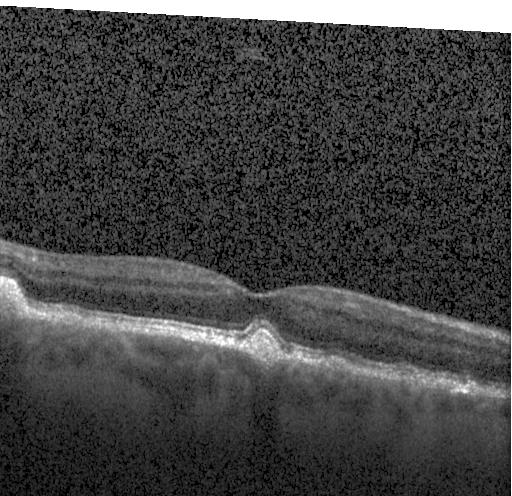

Heidelberg Spectralis OCT system. Optical coherence tomography B-scan. Spectral-domain OCT. Through the macula — The scan shows drusen.